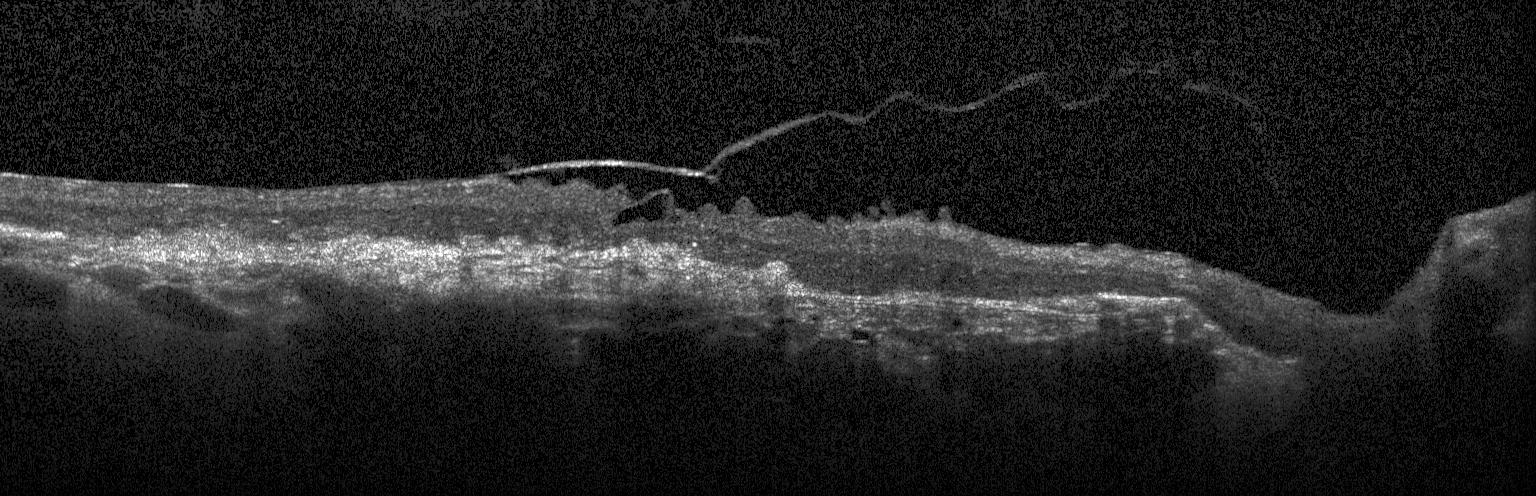

Dx: a choroidal neovascular membrane.